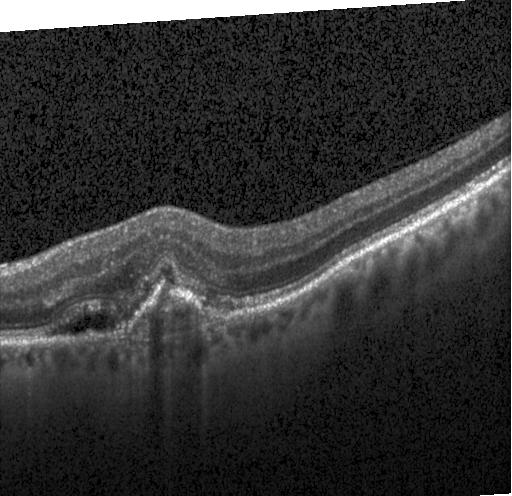
Heidelberg Spectralis, optical coherence tomography scan, centered on the fovea.
Impression: choroidal neovascularization.